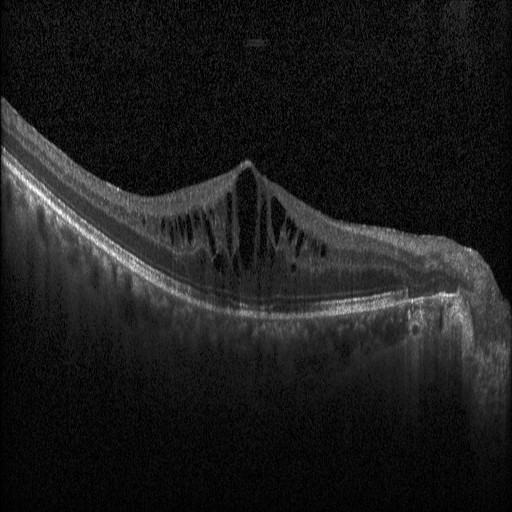 Spectral-domain optical coherence tomography, OCT line scan, Heidelberg Spectralis — Finding: diabetic macular edema (DME).